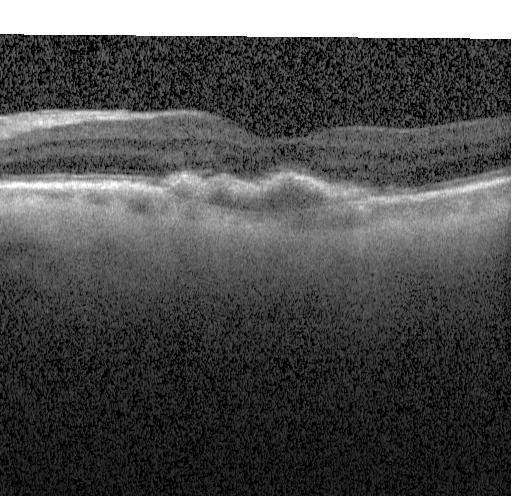

Retinal OCT B-scan; centered on the fovea; spectral-domain optical coherence tomography; Heidelberg Spectralis.
Finding: choroidal neovascularization (CNV).